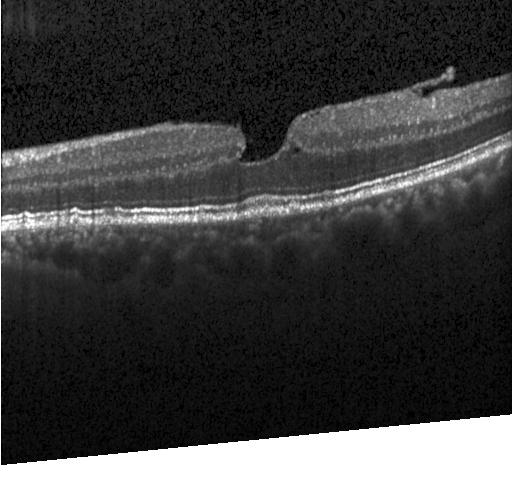 Retinal OCT cross-section.
Macular OCT: multiple drusen.